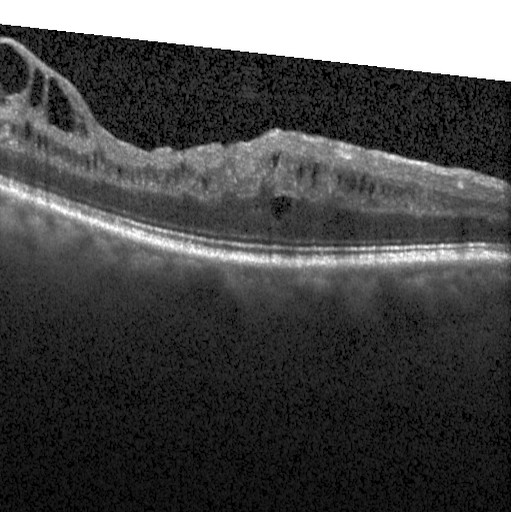 Finding: diabetic macular edema.